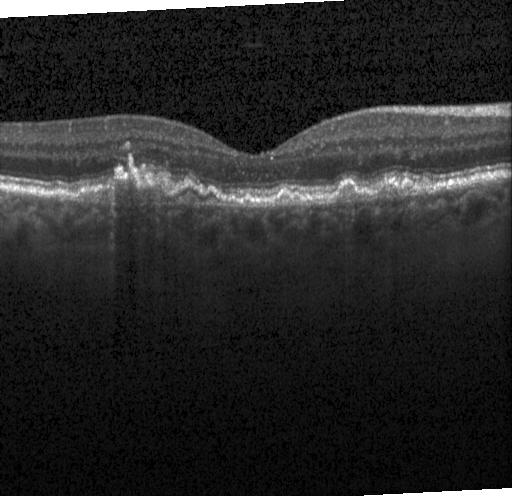
Optical coherence tomography scan.
Macular OCT: choroidal neovascularization (CNV).